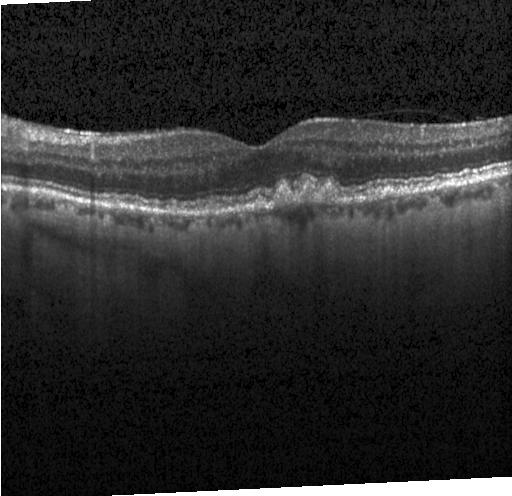

Macular OCT demonstrating drusen.